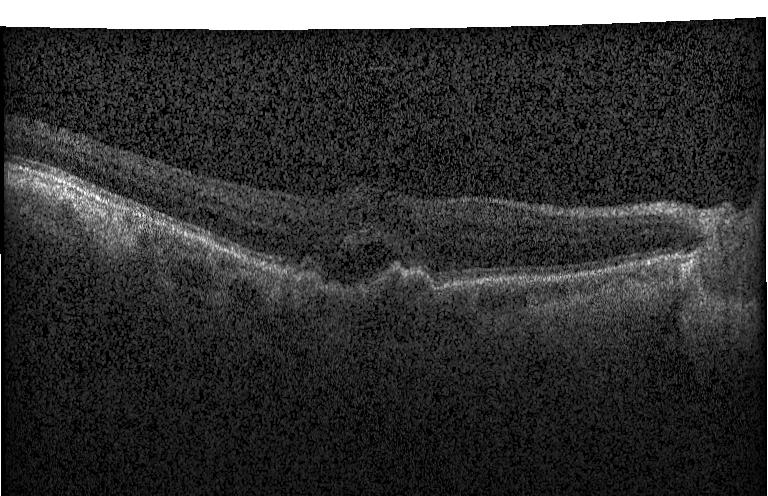 Instrument: Heidelberg Spectralis. OCT B-scan. Finding: a choroidal neovascular membrane.